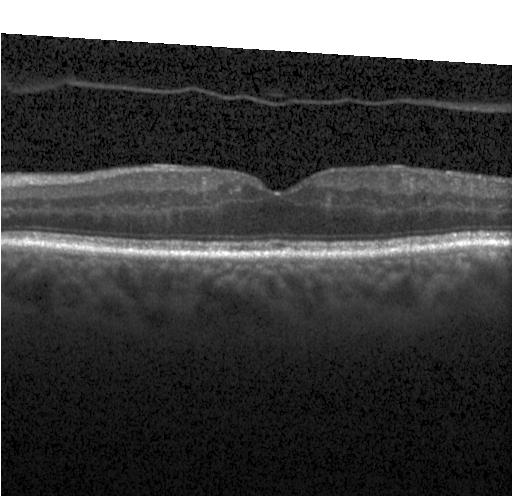
OCT scan showing no choroidal neovascularization, no diabetic macular edema, and no drusen.